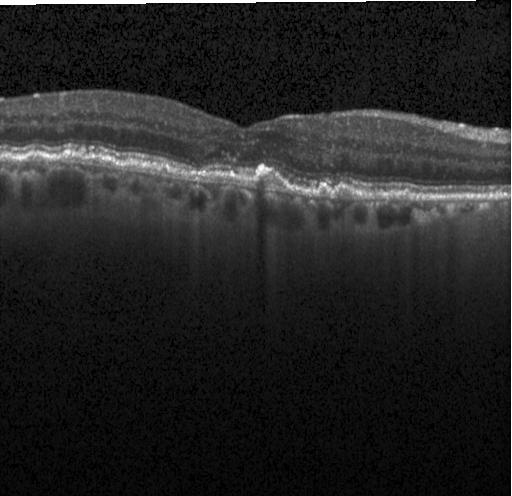
Impression: choroidal neovascularization.